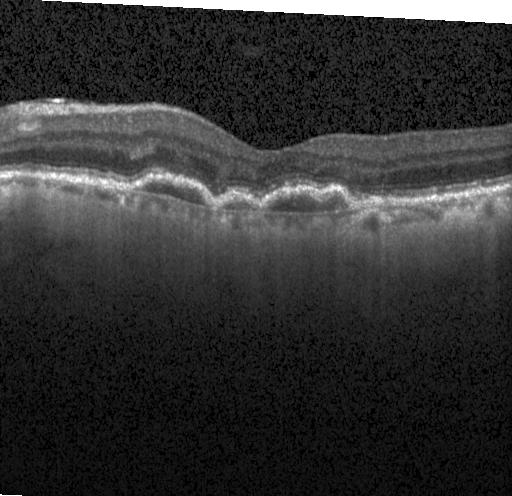 Optical coherence tomography B-scan
Finding: a choroidal neovascular membrane.